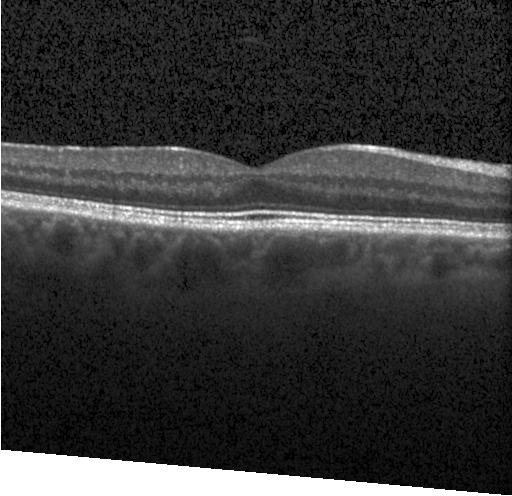
Neither CNV, DME, nor drusen.